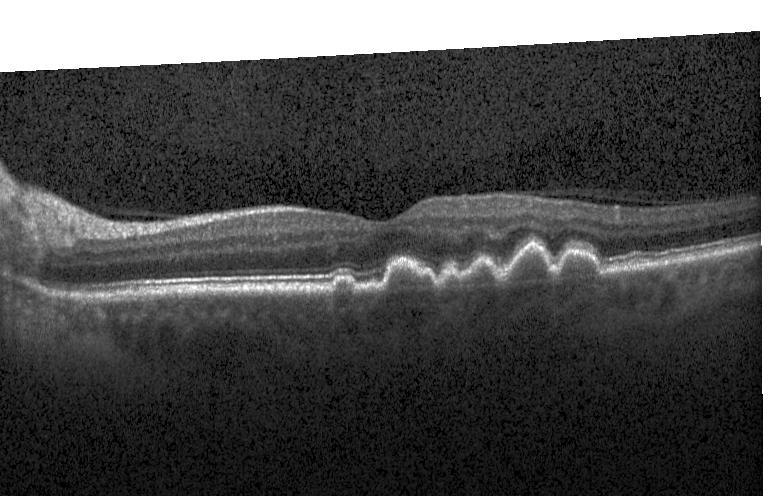 Optical coherence tomography scan. The scan shows drusen.